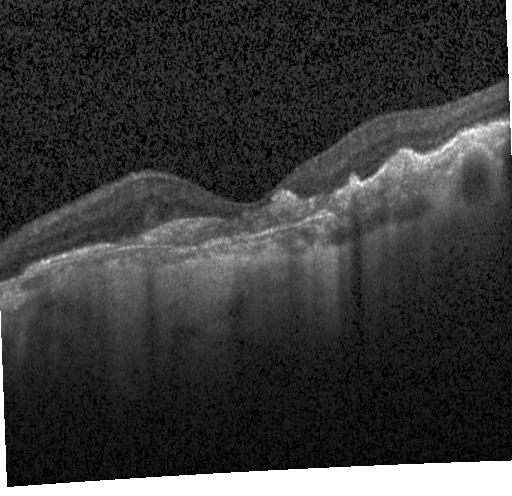 Instrument: Heidelberg Spectralis. OCT B-scan. Impression: a choroidal neovascular membrane.